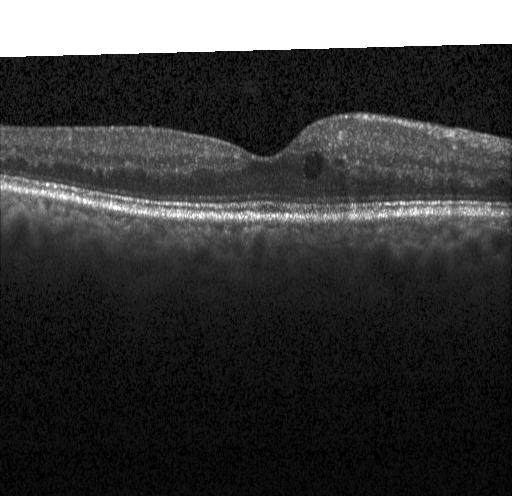

OCT line scan
Finding: DME.